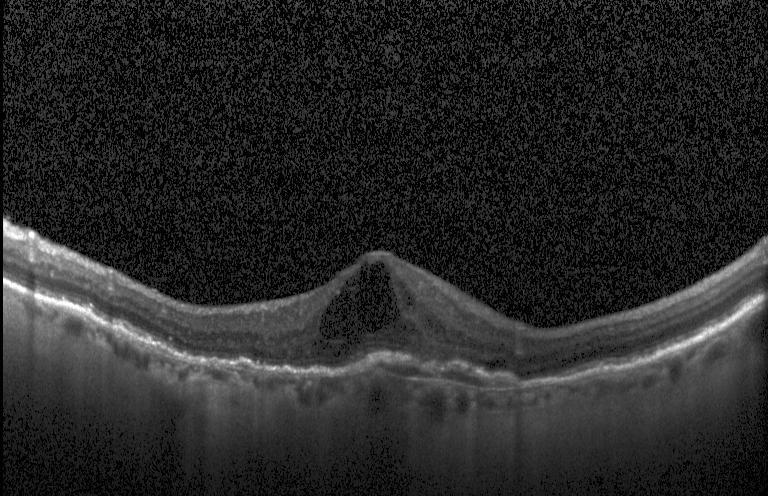
Optical coherence tomography B-scan — This B-scan demonstrates choroidal neovascularization (CNV).